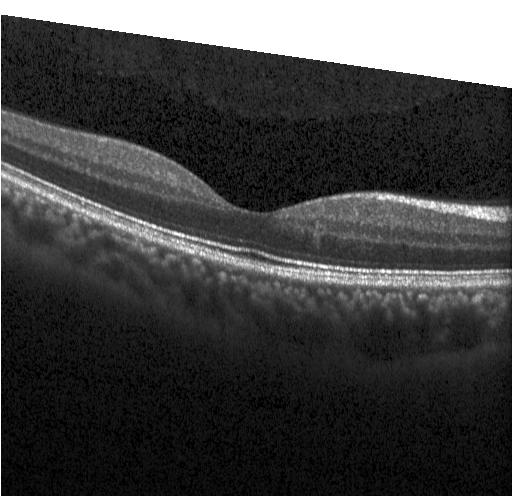
Retinal OCT B-scan. Heidelberg Spectralis OCT system. Spectral-domain OCT — Assessment: no choroidal neovascularization, diabetic macular edema, or drusen.